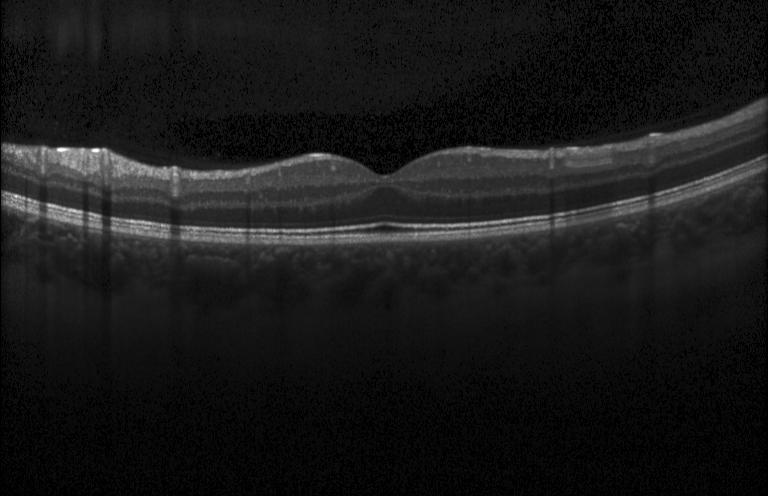 Retinal OCT B-scan. Diagnosis: no choroidal neovascularization, diabetic macular edema, or drusen.